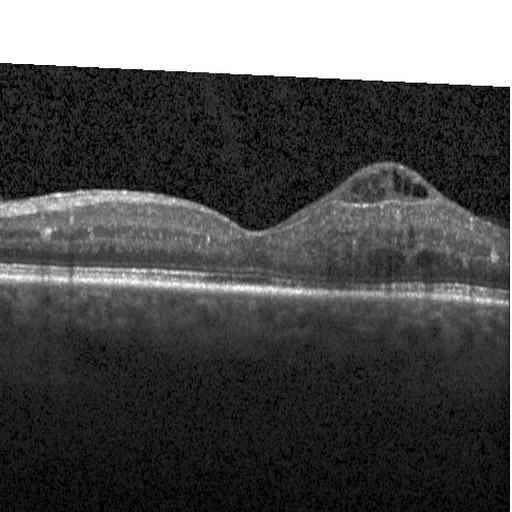

Heidelberg Spectralis OCT system · retinal OCT B-scan. Diagnosis: diabetic macular edema (DME).